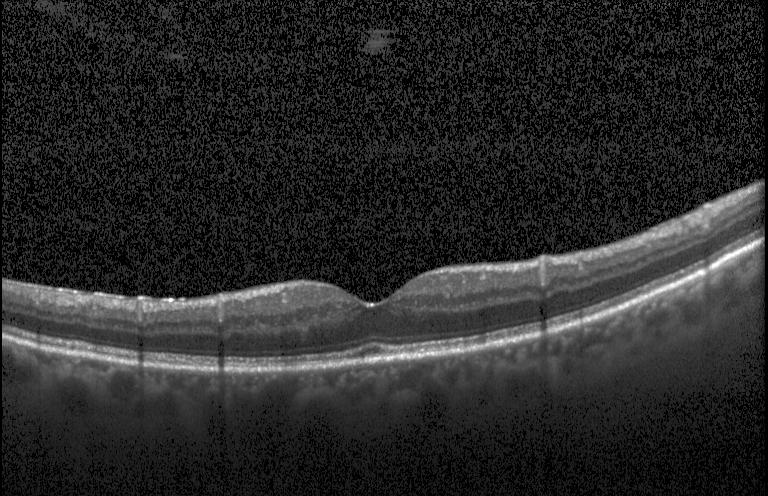 SD-OCT, acquired on a Heidelberg Spectralis, OCT B-scan. Diagnosis: no choroidal neovascularization, no diabetic macular edema, and no drusen.